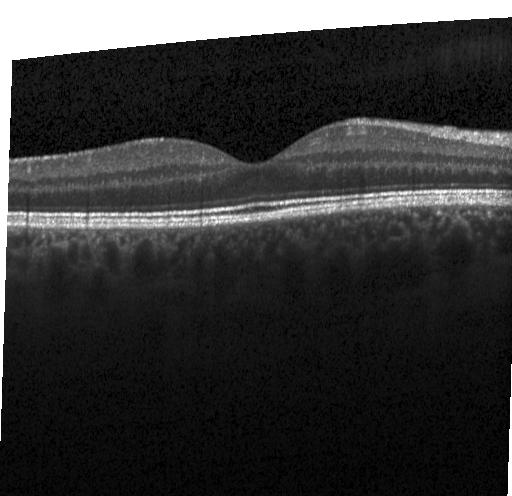

Optical coherence tomography B-scan.
OCT finding: neither choroidal neovascularization, diabetic macular edema, nor drusen.